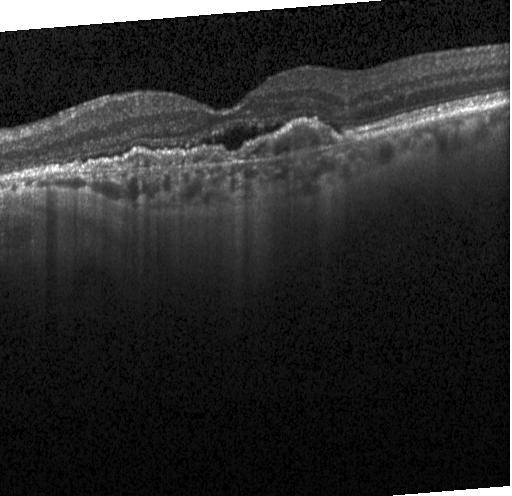
Retinal OCT cross-section · Heidelberg Spectralis · spectral-domain optical coherence tomography · centered on the fovea — Finding: choroidal neovascularization (CNV).